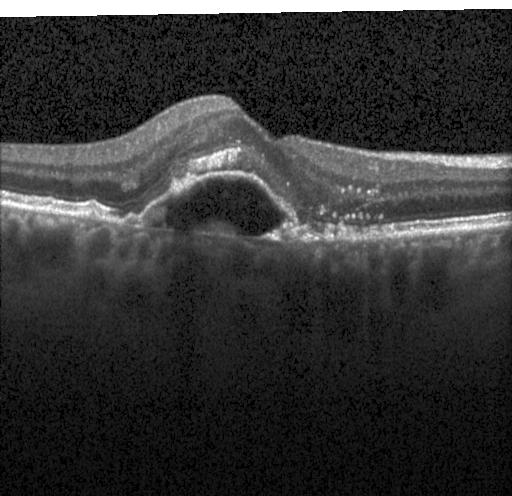
Heidelberg Spectralis OCT system. Optical coherence tomography B-scan. Fovea-centered. SD-OCT.
Diagnosis: choroidal neovascularization.